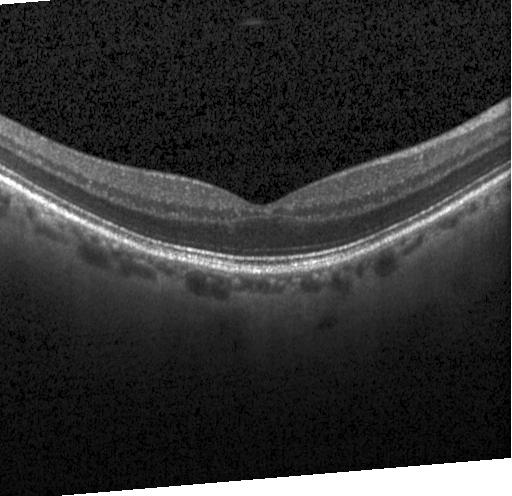

Impression: neither CNV, DME, nor drusen.